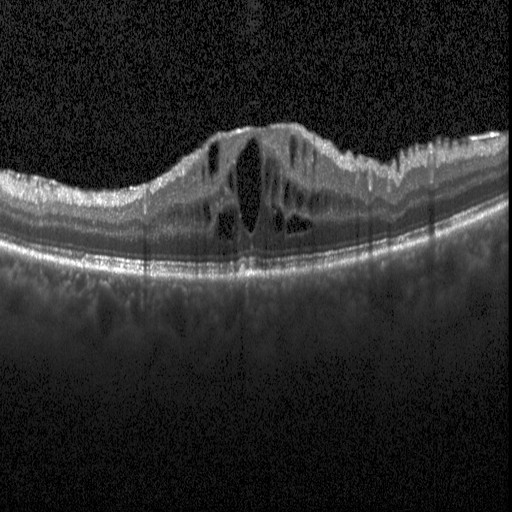 This B-scan demonstrates diabetic macular edema (DME).